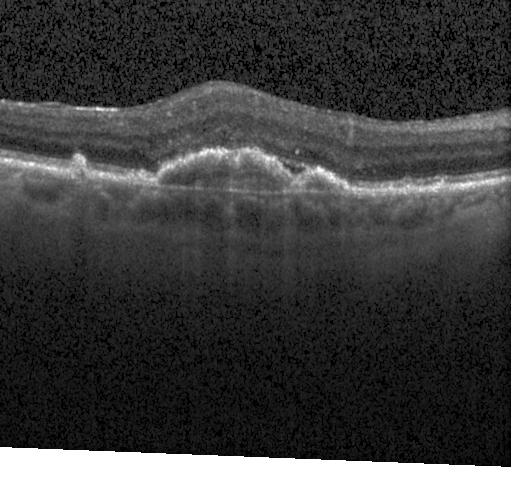

Macular scan. Acquired on a Heidelberg Spectralis. Optical coherence tomography B-scan
Finding: a choroidal neovascular membrane.